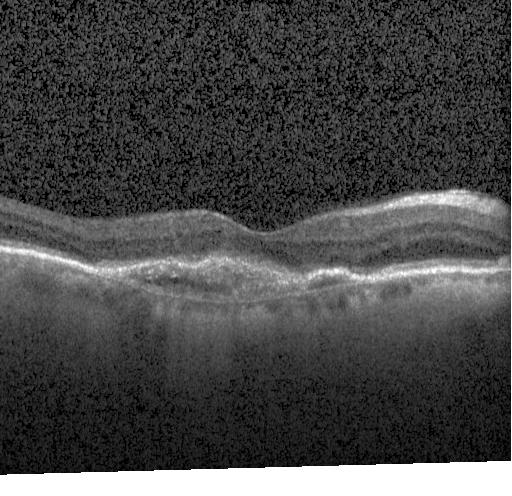
Acquired on a Heidelberg Spectralis. Spectral-domain optical coherence tomography. Optical coherence tomography scan. Centered on the fovea.
The scan shows CNV.